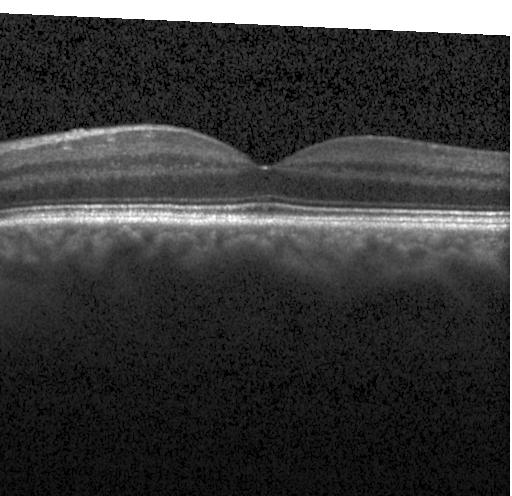 Retinal OCT cross-section. Through the macula. Heidelberg Spectralis.
Neither choroidal neovascularization, diabetic macular edema, nor drusen.